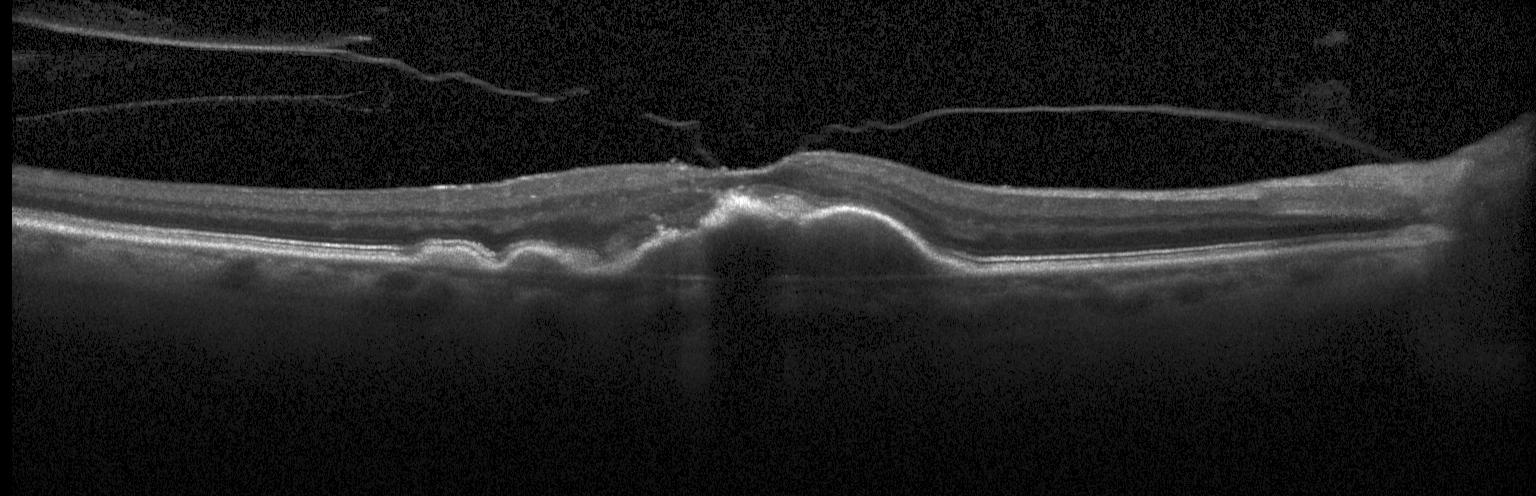

OCT B-scan — This B-scan demonstrates choroidal neovascularization (CNV).